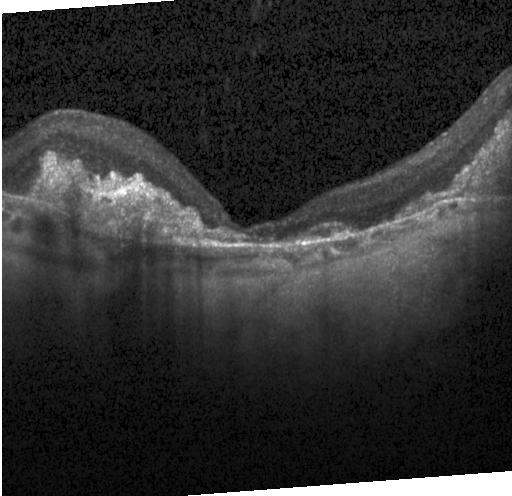

Retinal OCT cross-section. Spectral-domain optical coherence tomography. Acquired on a Heidelberg Spectralis — Macular OCT: choroidal neovascularization (CNV).